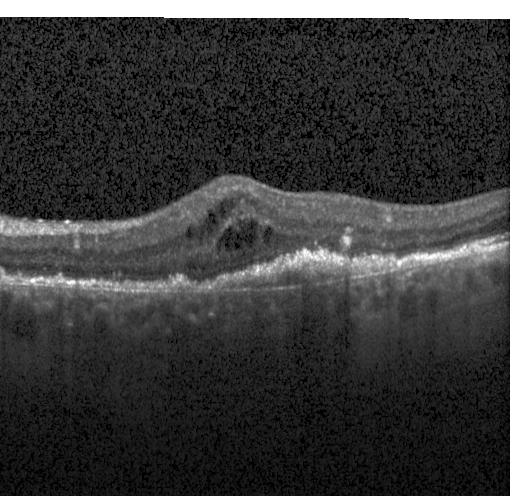 Horizontal scan through the fovea. SD-OCT. Heidelberg Spectralis. OCT B-scan.
Diagnosis: a choroidal neovascular membrane.